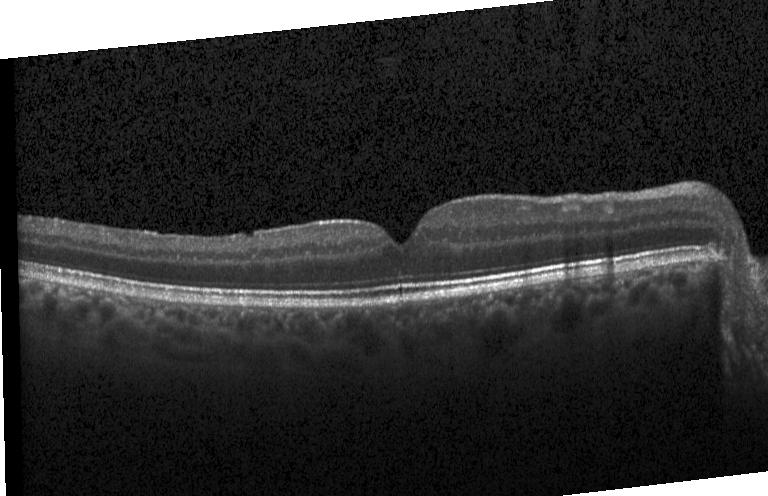
Dx: no choroidal neovascularization, no diabetic macular edema, and no drusen.